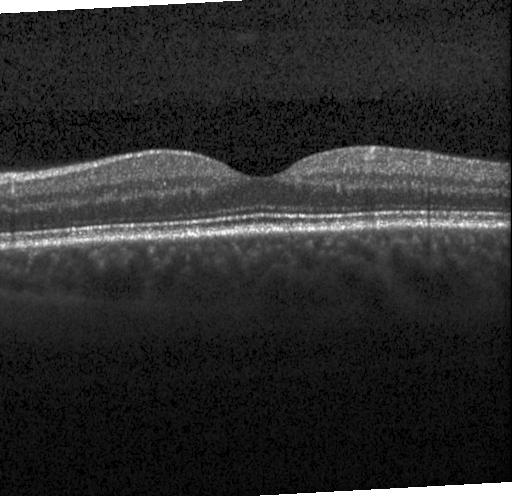 Retinal OCT B-scan, spectral-domain optical coherence tomography.
Macular OCT: neither choroidal neovascularization, diabetic macular edema, nor drusen.